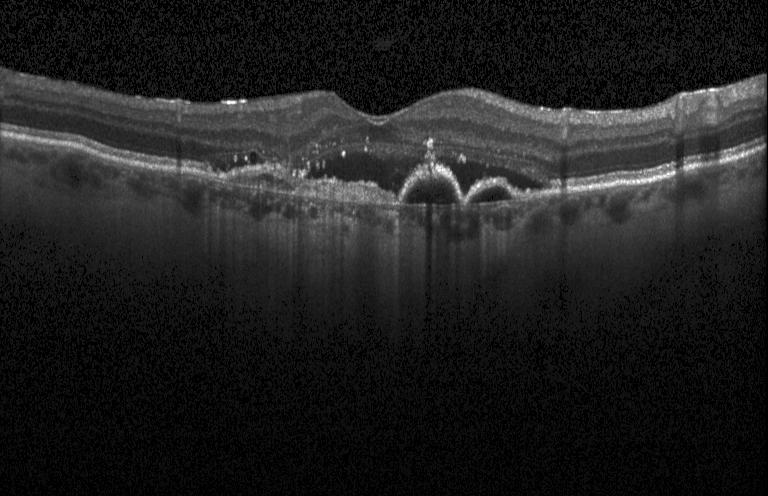 Optical coherence tomography B-scan · spectral-domain OCT · horizontal scan through the fovea · Heidelberg Spectralis OCT system. Impression: choroidal neovascularization.